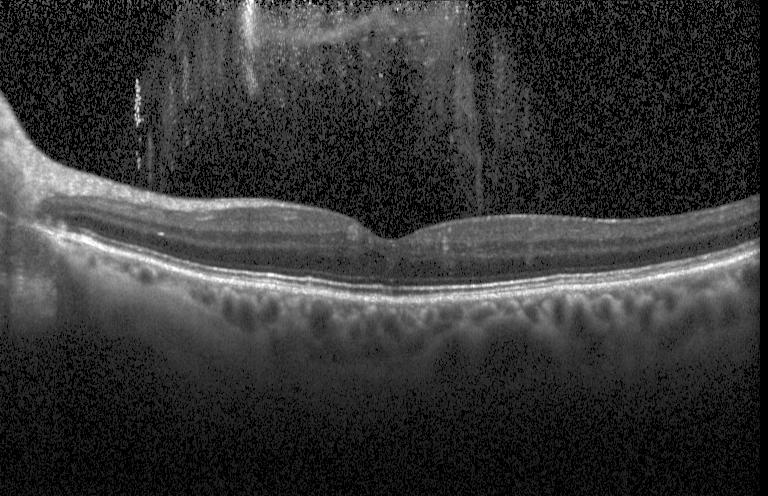 Macular scan. Optical coherence tomography B-scan. Acquired on a Heidelberg Spectralis
Diagnosis: no CNV, DME, or drusen.